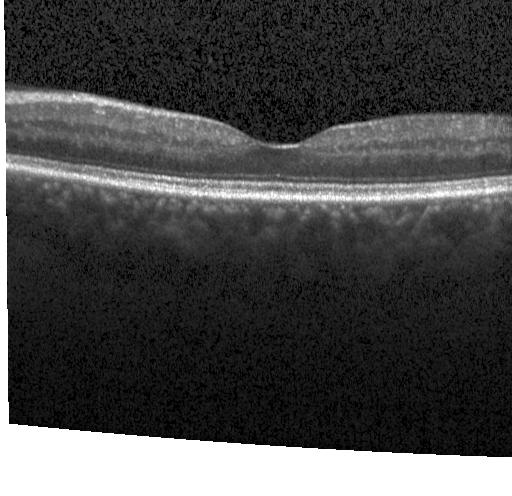 Spectral-domain OCT · horizontal scan through the fovea · OCT B-scan
Assessment: no choroidal neovascularization, no diabetic macular edema, and no drusen.